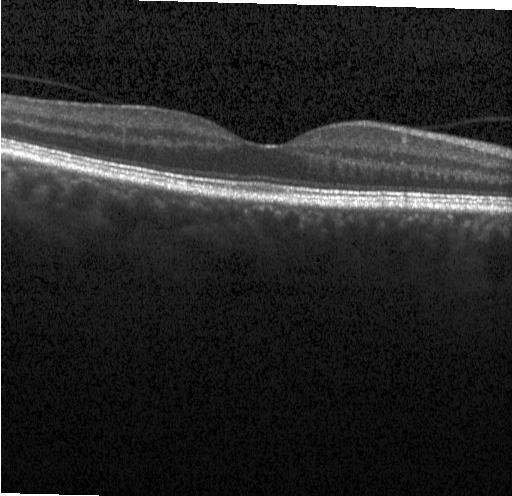
Retinal OCT B-scan
Impression: no choroidal neovascularization, no diabetic macular edema, and no drusen.